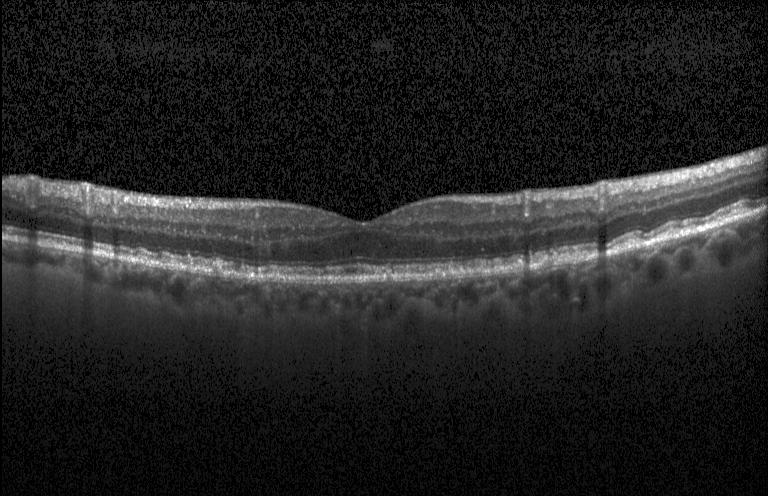

Horizontal scan through the fovea. Instrument: Heidelberg Spectralis. Retinal OCT B-scan.
Assessment: sub-RPE drusenoid deposits.